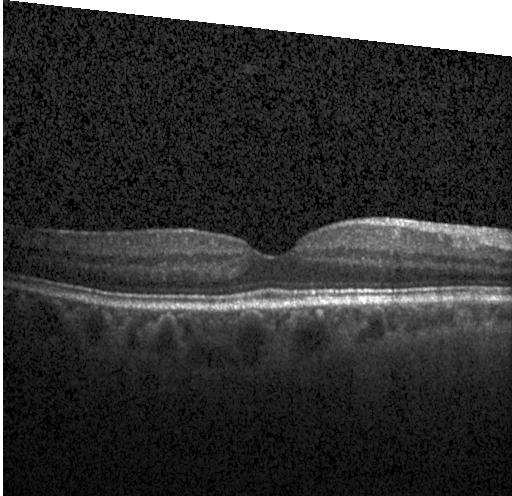
This B-scan demonstrates no evidence of choroidal neovascularization, diabetic macular edema, or drusen.